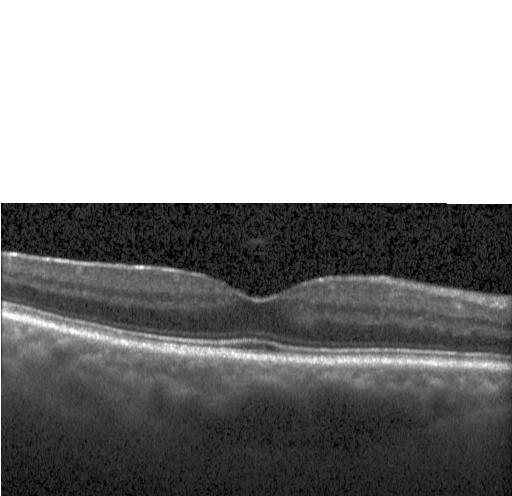

Neither choroidal neovascularization, diabetic macular edema, nor drusen.